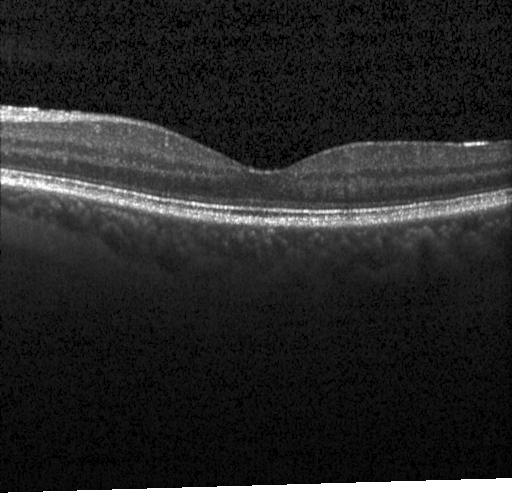
Heidelberg Spectralis; spectral-domain optical coherence tomography; macular scan; retinal OCT B-scan. Finding: no evidence of CNV, DME, or drusen.